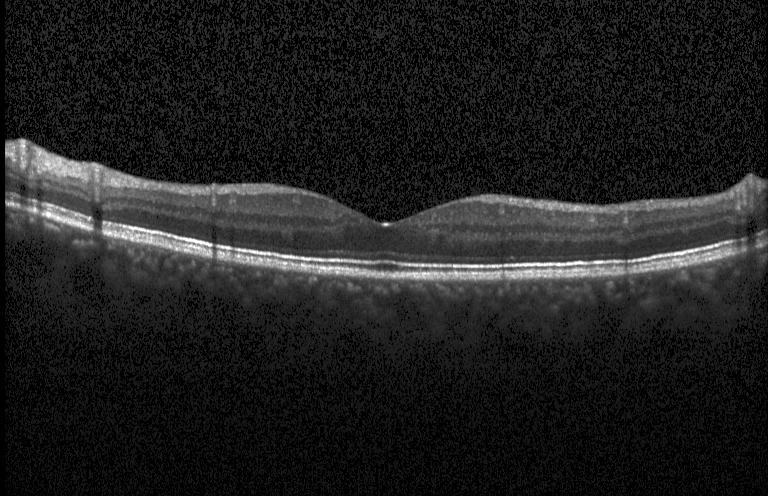
OCT line scan, Heidelberg Spectralis, spectral-domain optical coherence tomography.
Assessment: no choroidal neovascularization, no diabetic macular edema, and no drusen.